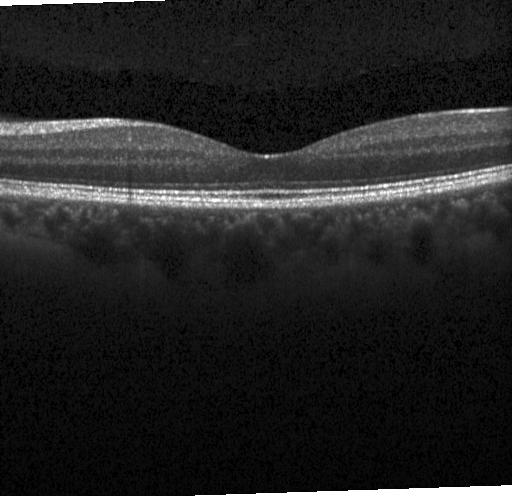
Retinal OCT cross-section. Impression: no CNV, no DME, and no drusen.